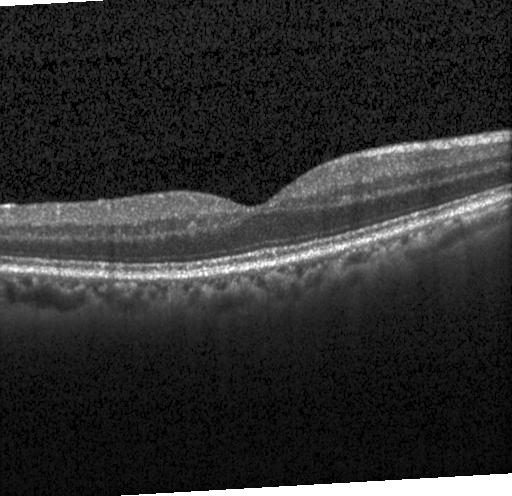

Optical coherence tomography B-scan · through the macula. Dx: no choroidal neovascularization, diabetic macular edema, or drusen.